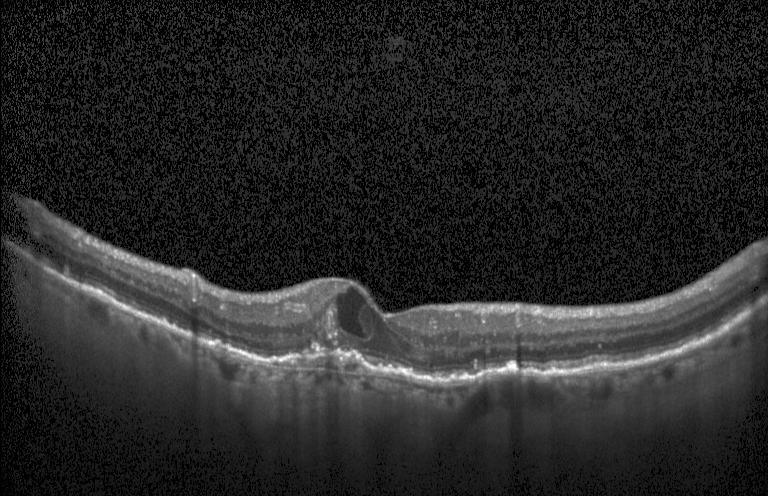
Macular OCT: choroidal neovascularization (CNV).